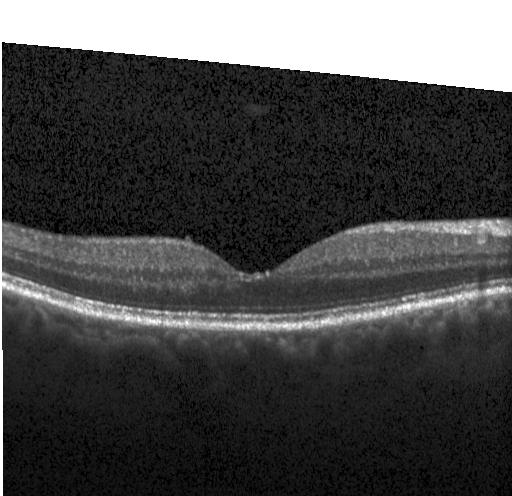 Assessment: no choroidal neovascularization, no diabetic macular edema, and no drusen.